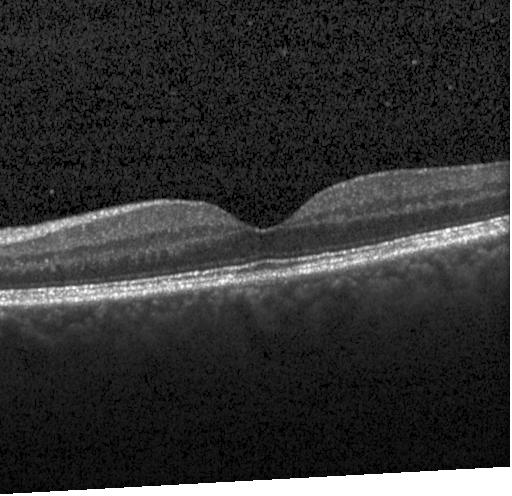

Retinal OCT B-scan; acquired on a Heidelberg Spectralis; spectral-domain optical coherence tomography; fovea-centered. The scan shows no choroidal neovascularization, no diabetic macular edema, and no drusen.